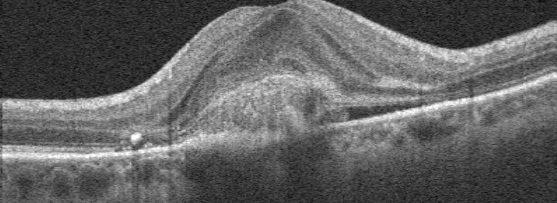
Macular OCT demonstrating age-related macular degeneration.